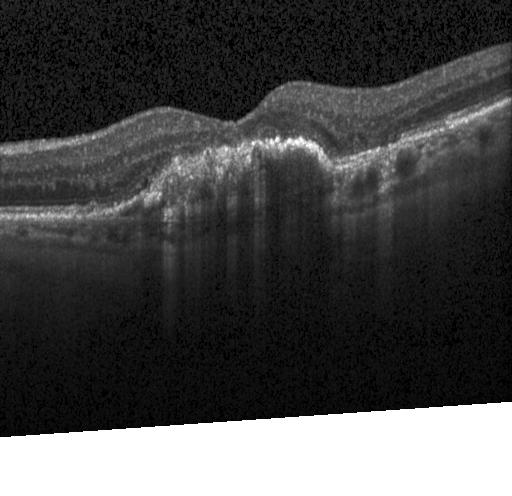
Retinal OCT cross-section · fovea-centered
Choroidal neovascularization.